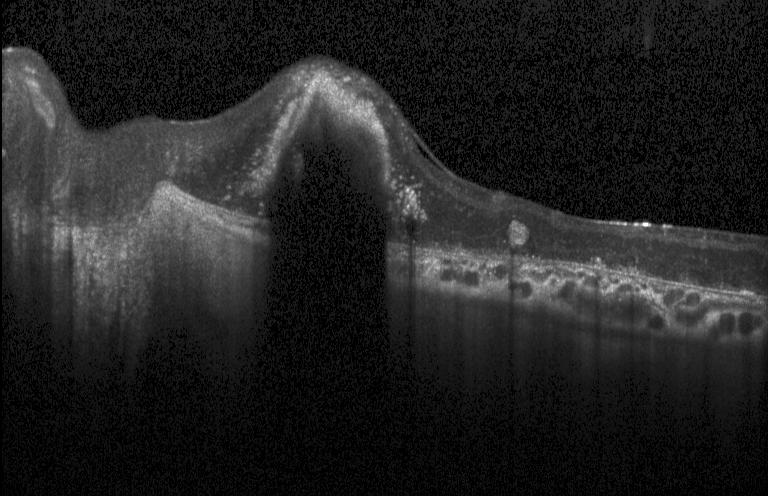 Retinal OCT cross-section showing a choroidal neovascular membrane.